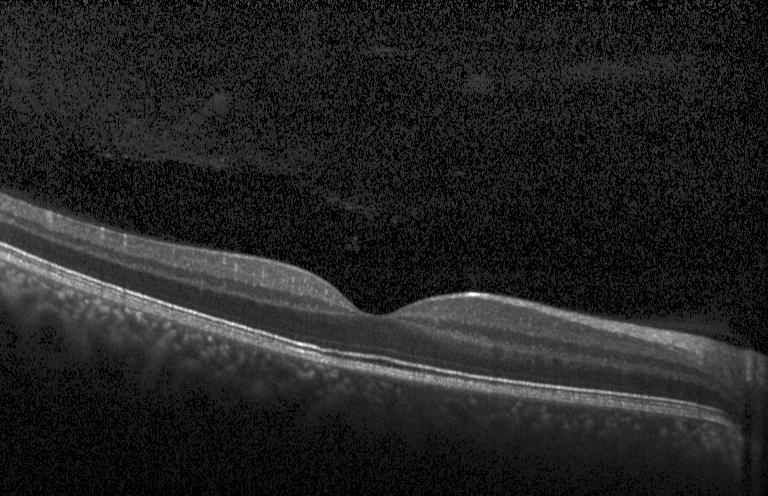
Heidelberg Spectralis · OCT line scan · SD-OCT.
Impression: no choroidal neovascularization, no diabetic macular edema, and no drusen.